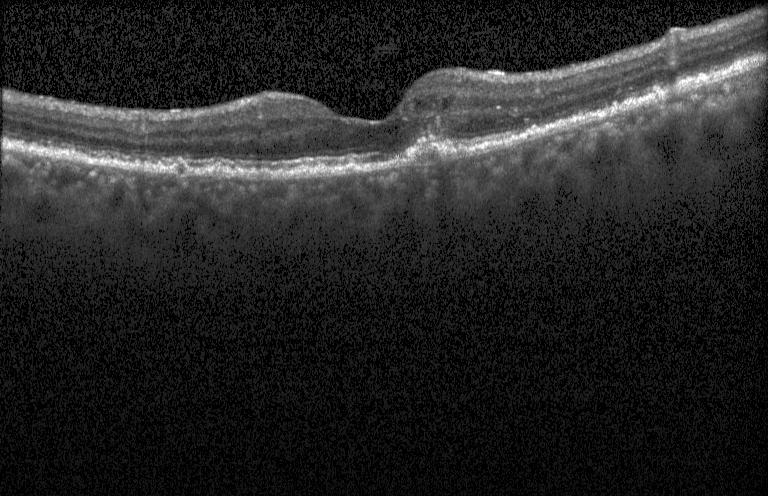

A choroidal neovascular membrane.